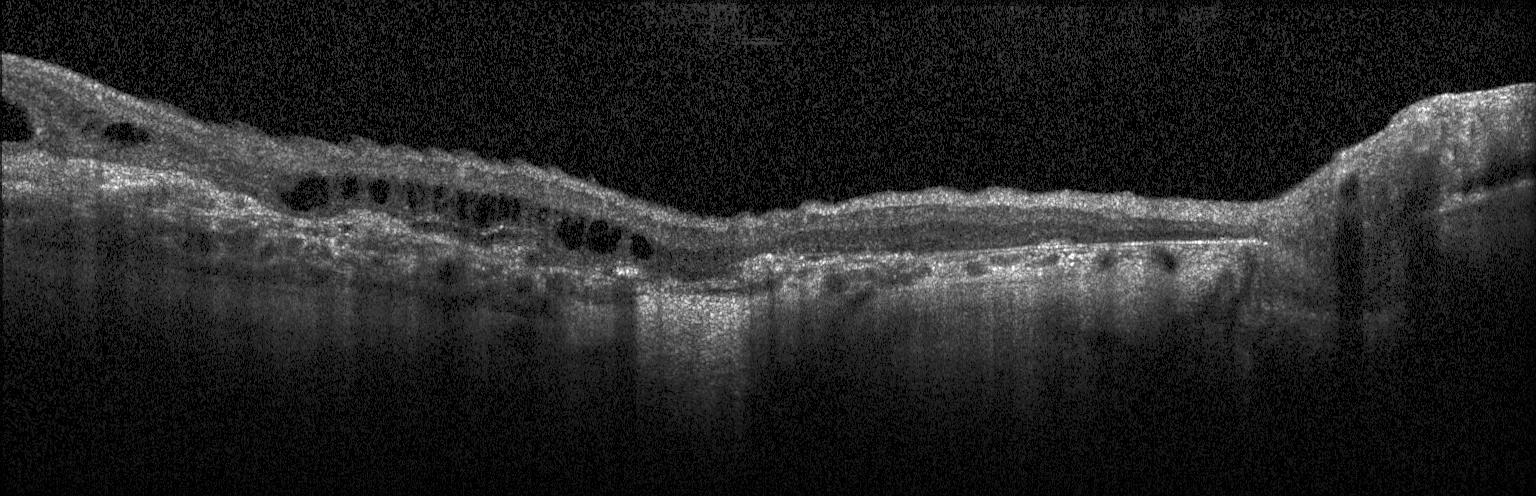
Macular OCT: a choroidal neovascular membrane.